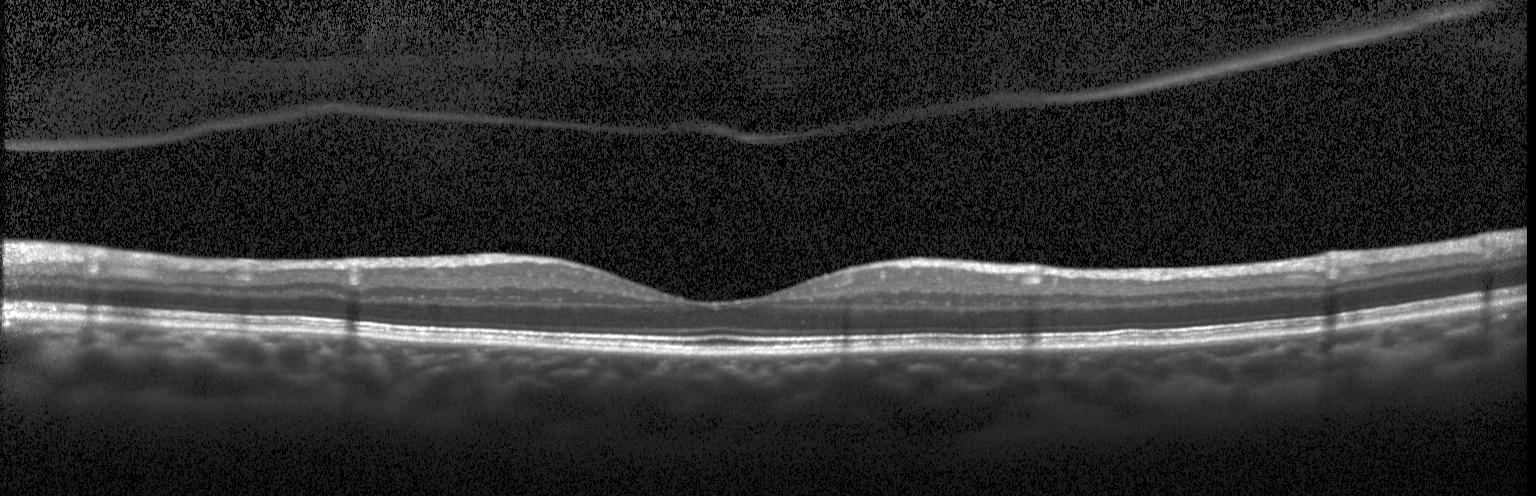

Retinal OCT cross-section showing no CNV, DME, or drusen.